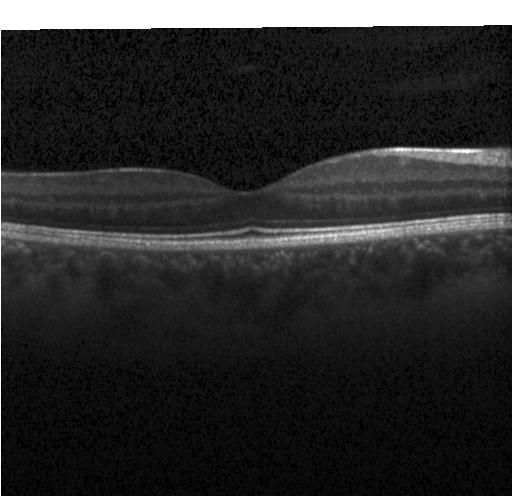
Spectral-domain optical coherence tomography; retinal OCT B-scan; Heidelberg Spectralis.
Assessment: neither choroidal neovascularization, diabetic macular edema, nor drusen.